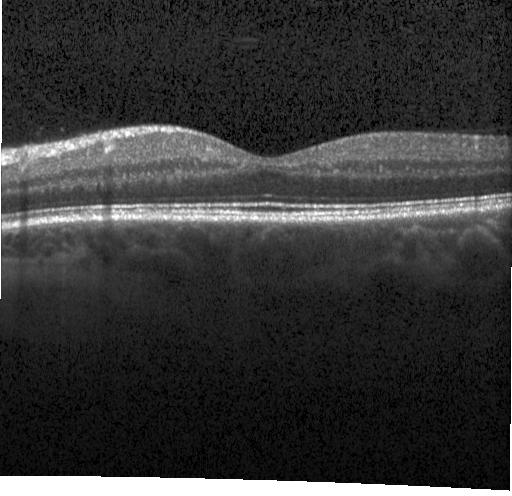
Retinal OCT cross-section, acquired on a Heidelberg Spectralis. No CNV, DME, or drusen.